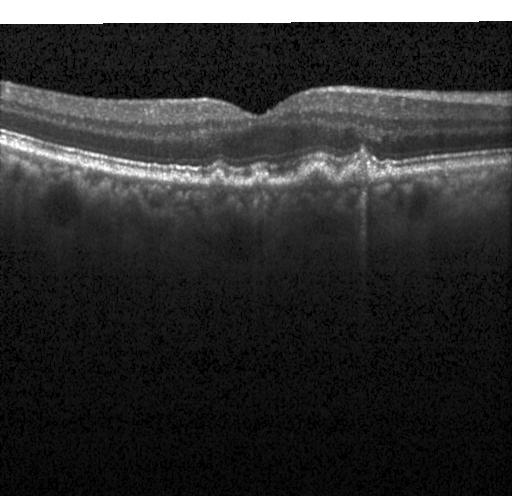

OCT line scan. Finding: sub-RPE drusenoid deposits.